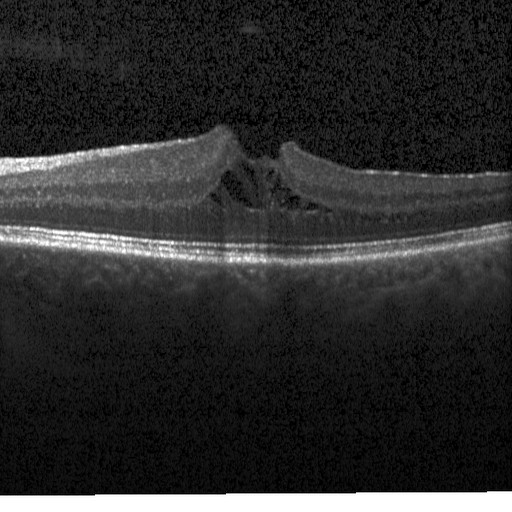 Optical coherence tomography scan, Heidelberg Spectralis OCT system, spectral-domain optical coherence tomography, fovea-centered.
Macular OCT: diabetic macular edema (DME).